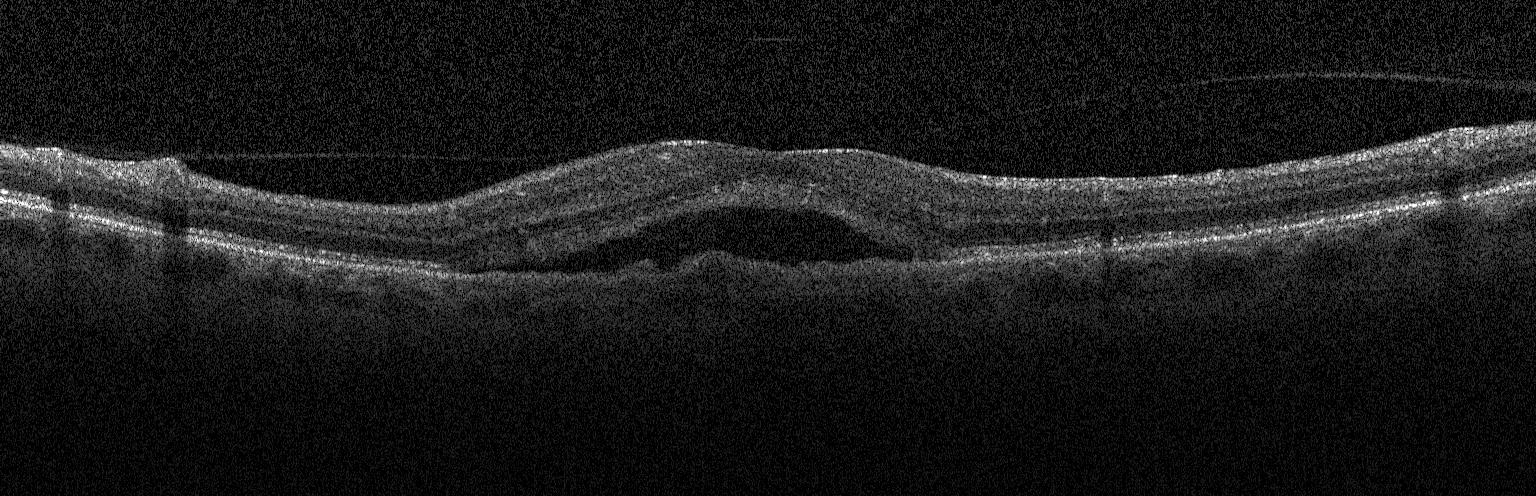 Acquired on a Heidelberg Spectralis; retinal OCT cross-section; spectral-domain optical coherence tomography; centered on the fovea — Impression: a choroidal neovascular membrane.